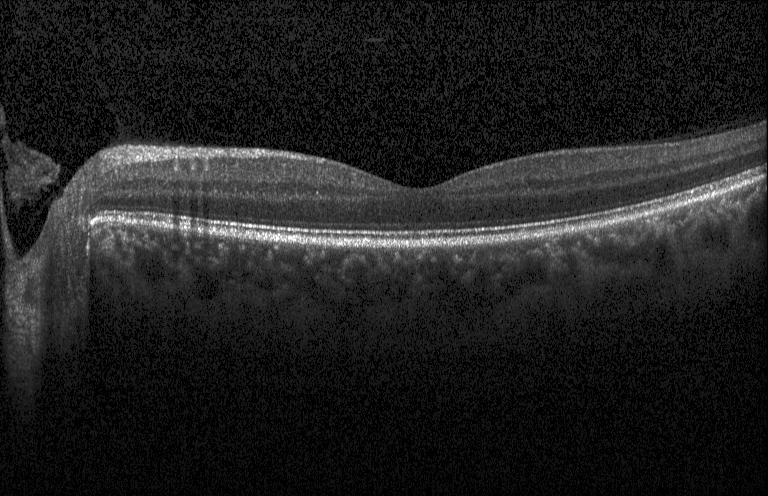 Finding: no choroidal neovascularization, diabetic macular edema, or drusen.